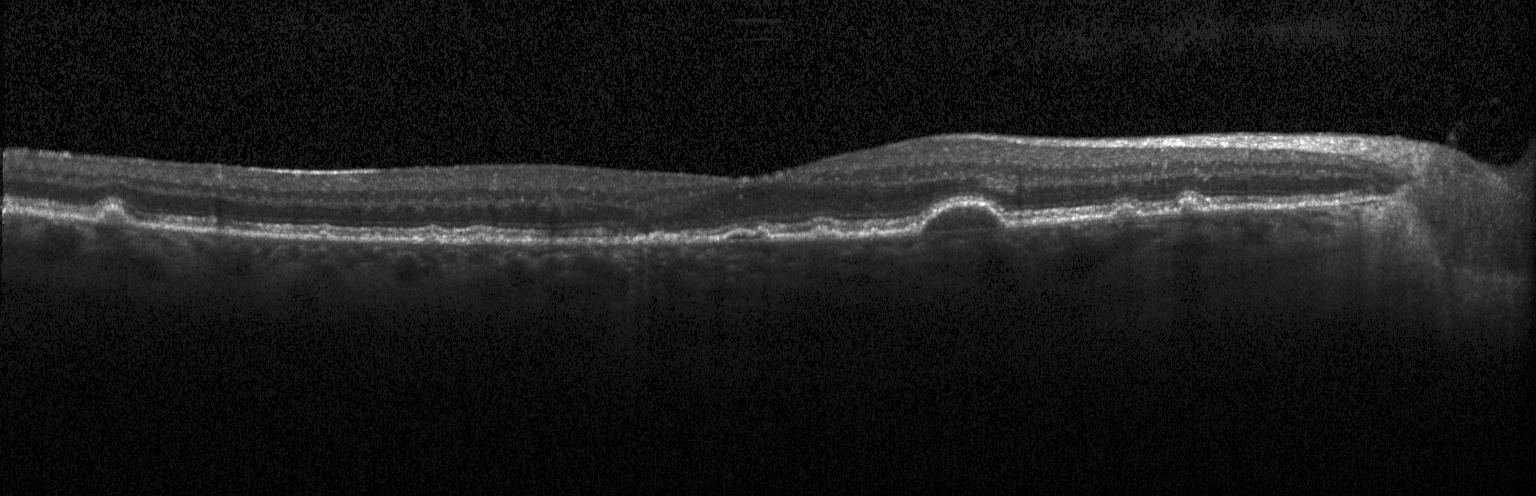

This B-scan demonstrates multiple drusen.